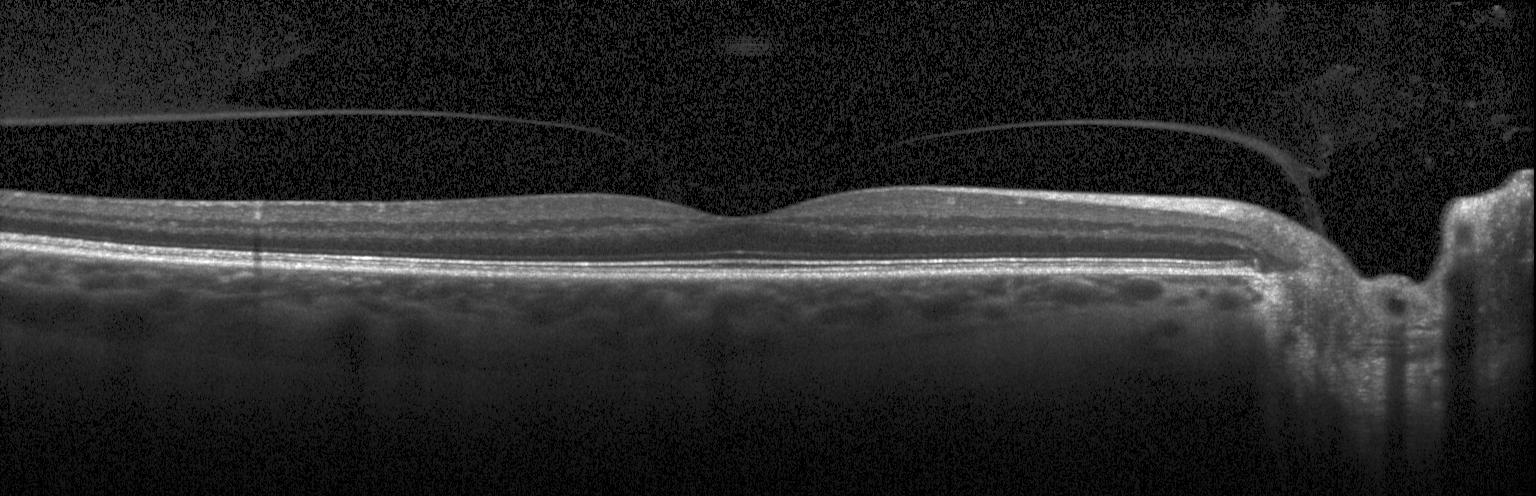 Instrument: Heidelberg Spectralis, fovea-centered, optical coherence tomography B-scan — Impression: no evidence of choroidal neovascularization, diabetic macular edema, or drusen.